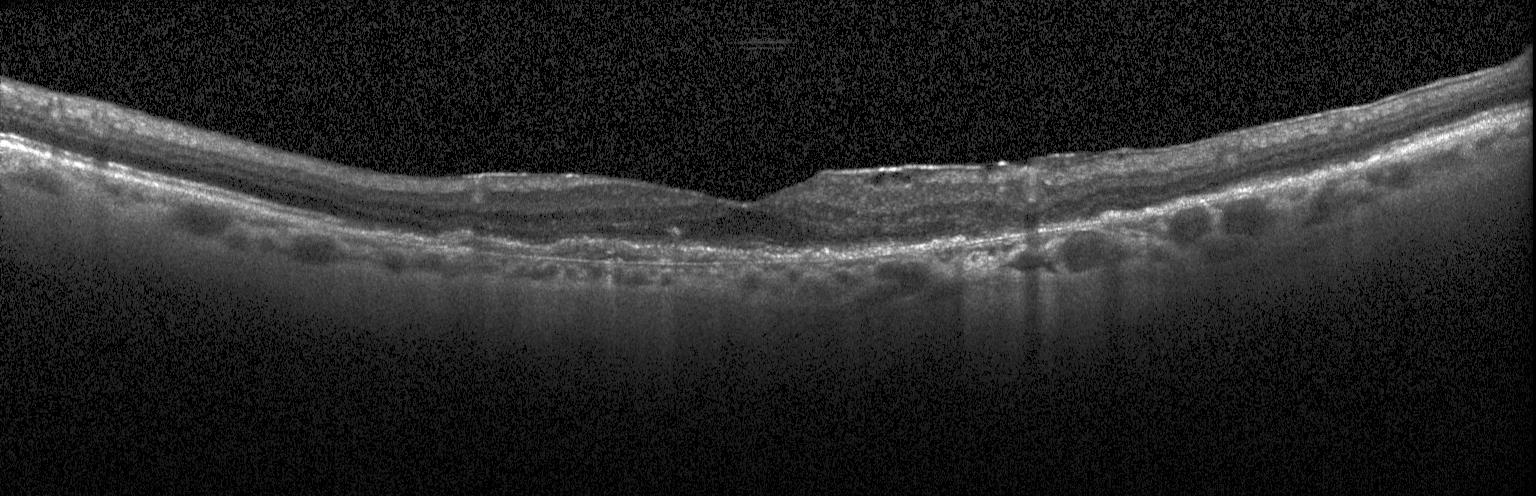
Optical coherence tomography scan. SD-OCT. Acquired on a Heidelberg Spectralis. Horizontal scan through the fovea.
A choroidal neovascular membrane.